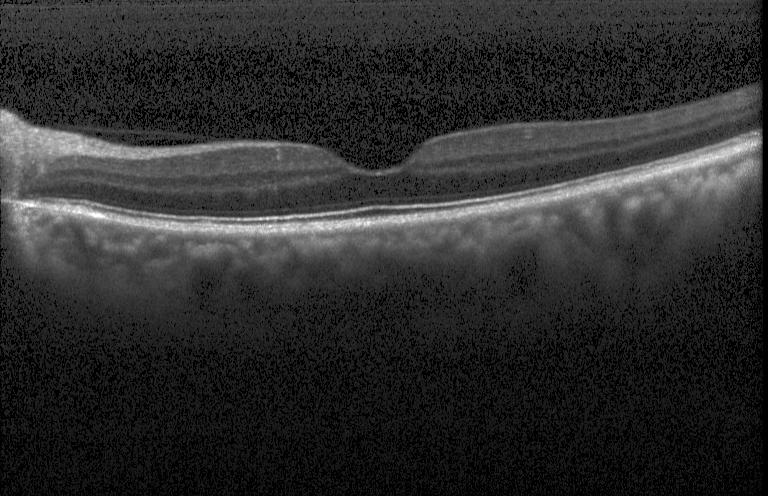

Diagnosis: no CNV, DME, or drusen.